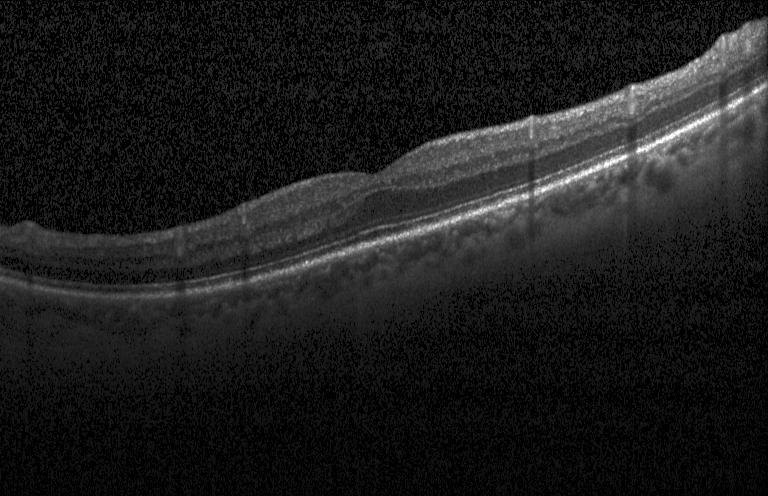
Acquired on a Heidelberg Spectralis, SD-OCT, retinal OCT cross-section
Assessment: no choroidal neovascularization, no diabetic macular edema, and no drusen.